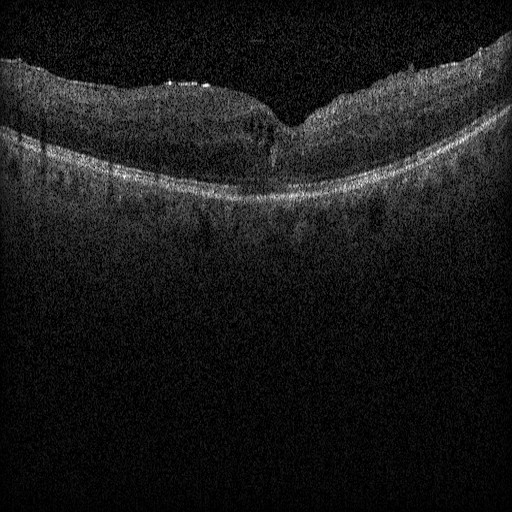
Spectral-domain optical coherence tomography; OCT line scan.
The scan shows diabetic macular edema.